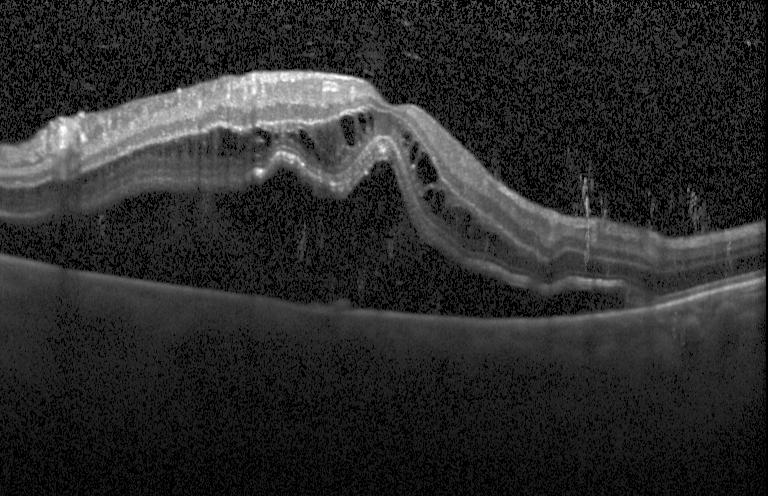

Centered on the fovea, SD-OCT, acquired on a Heidelberg Spectralis, retinal OCT B-scan.
Finding: diabetic macular edema (DME).